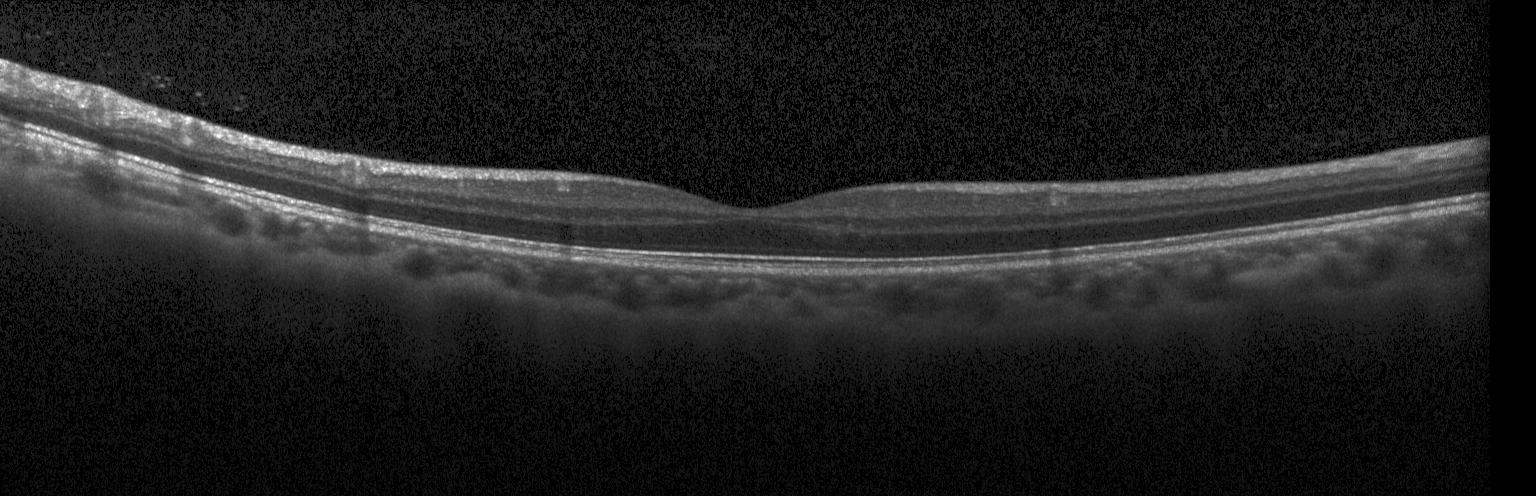

Diagnosis: no choroidal neovascularization, no diabetic macular edema, and no drusen.